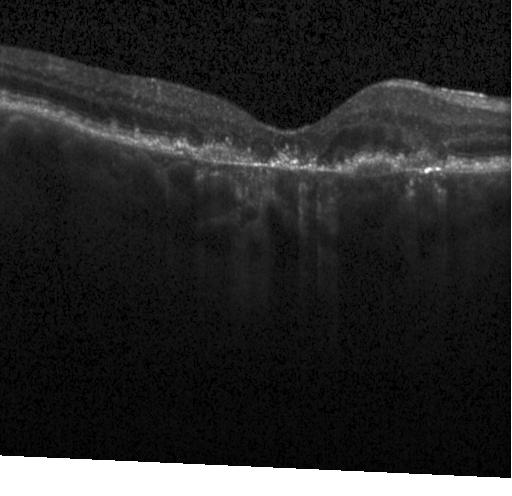 Retinal OCT cross-section.
Finding: choroidal neovascularization (CNV).